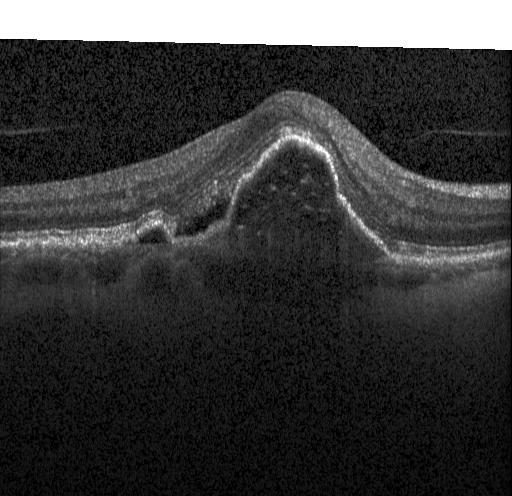
Optical coherence tomography scan. Macular OCT: choroidal neovascularization (CNV).